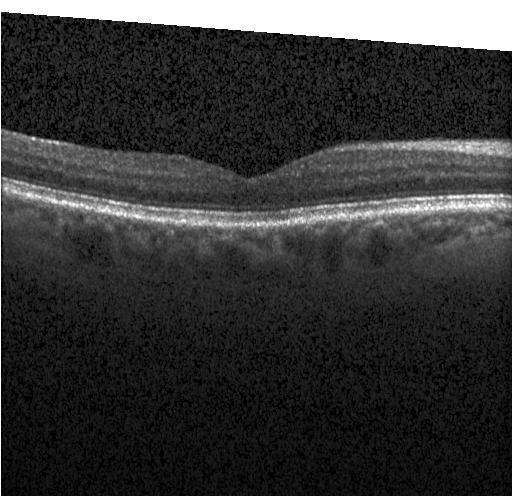
Macular OCT: no evidence of choroidal neovascularization, diabetic macular edema, or drusen.